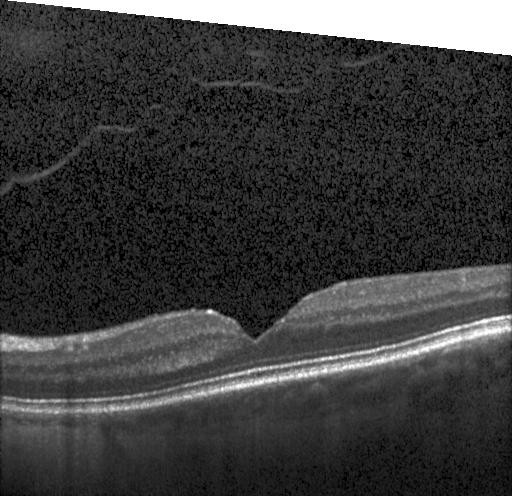
Diagnosis: no CNV, no DME, and no drusen.